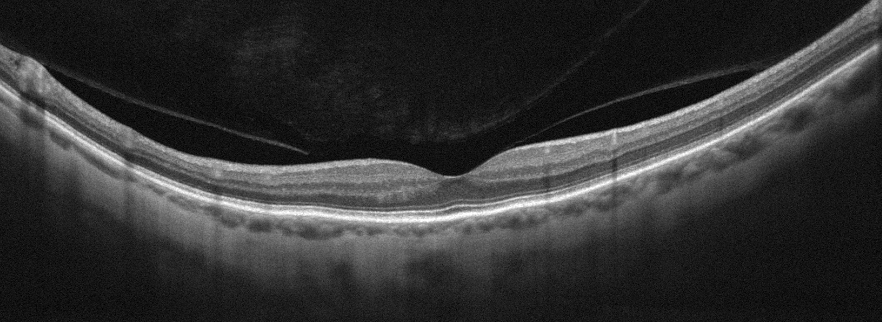

Acquired on an Optovue Avanti RTVue XR · OCT line scan · macular scan — Assessment: no evidence of AMD, DME, ERM, RAO, RVO, or VID.